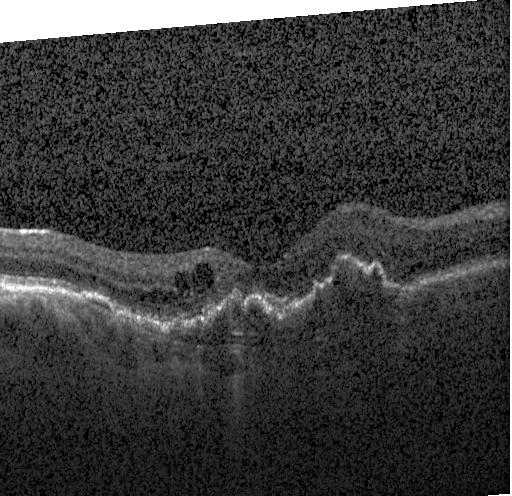
Macular OCT: a choroidal neovascular membrane.